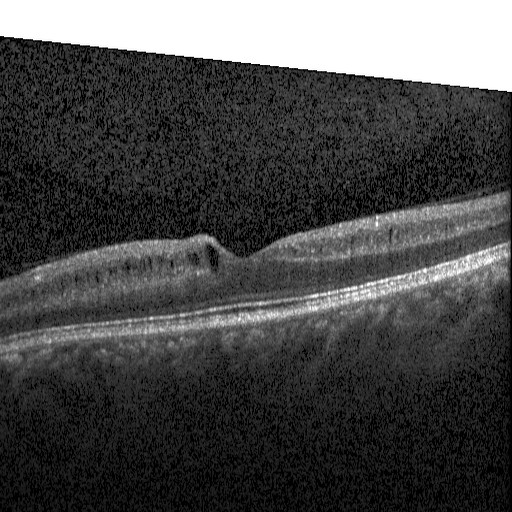
Heidelberg Spectralis OCT system · retinal OCT cross-section · centered on the fovea. Impression: DME.